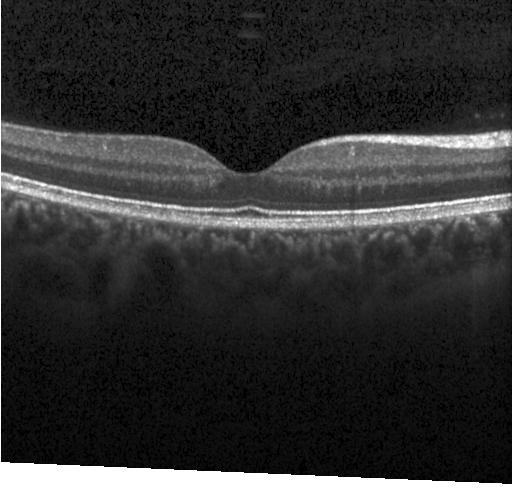

Optical coherence tomography B-scan
Macular OCT: no CNV, DME, or drusen.